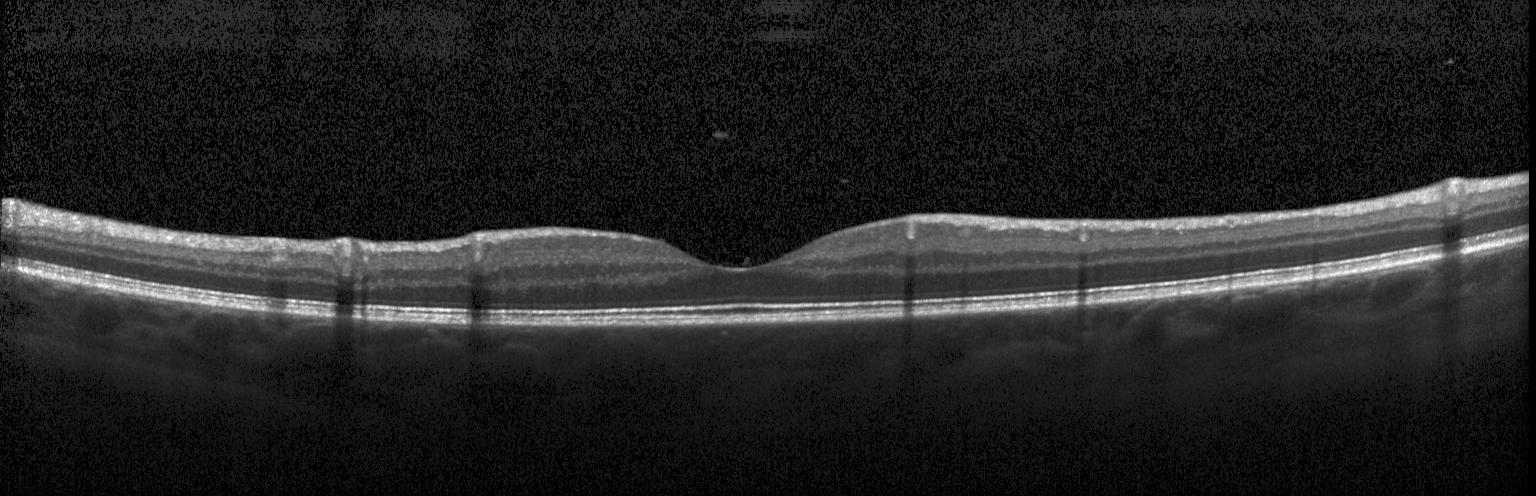
Optical coherence tomography B-scan. Dx: no choroidal neovascularization, diabetic macular edema, or drusen.